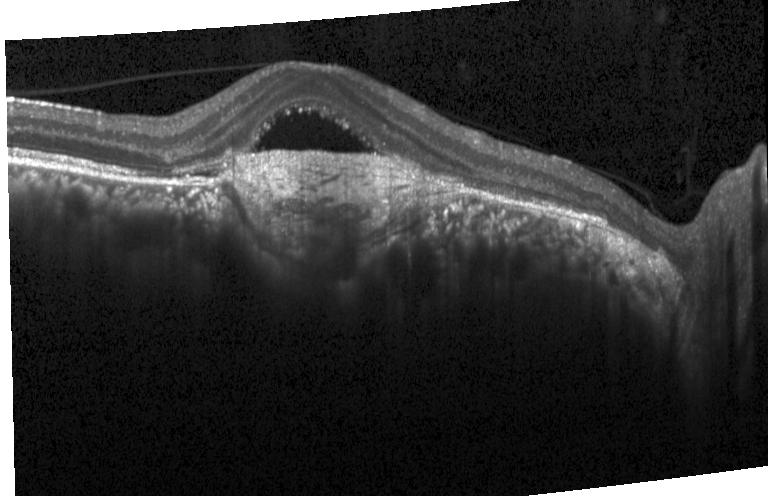
Horizontal scan through the fovea, retinal OCT B-scan
Diagnosis: CNV.